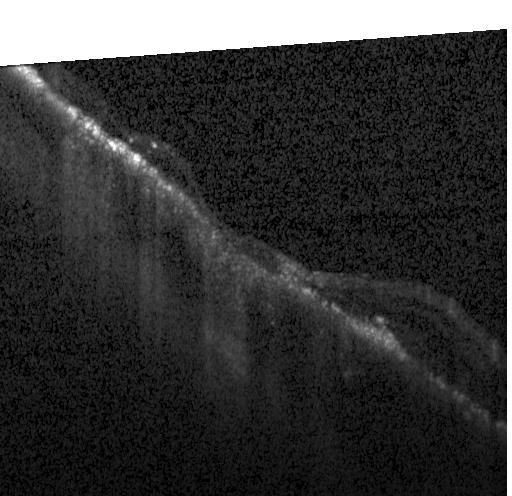
Retinal OCT cross-section showing a choroidal neovascular membrane.